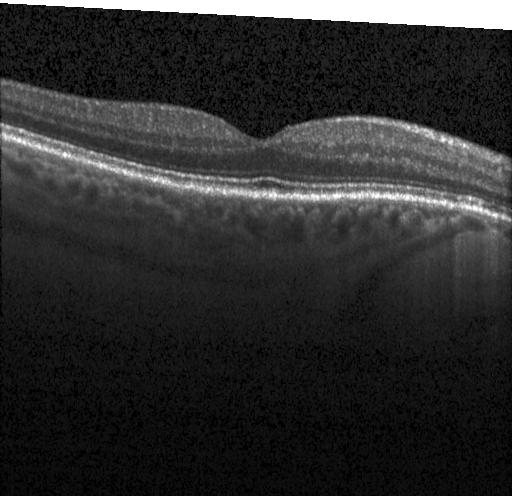

Optical coherence tomography B-scan
Finding: no CNV, no DME, and no drusen.